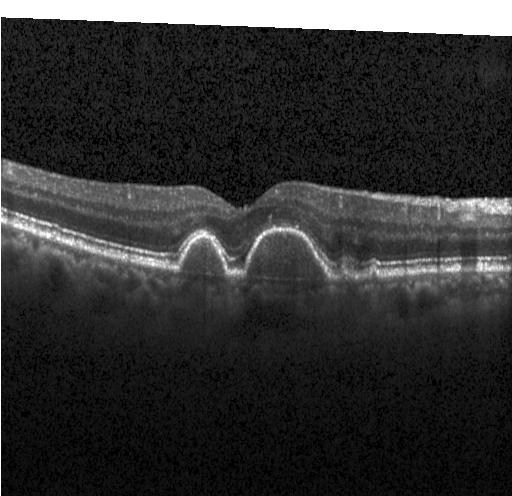

Optical coherence tomography B-scan
The scan shows drusen.